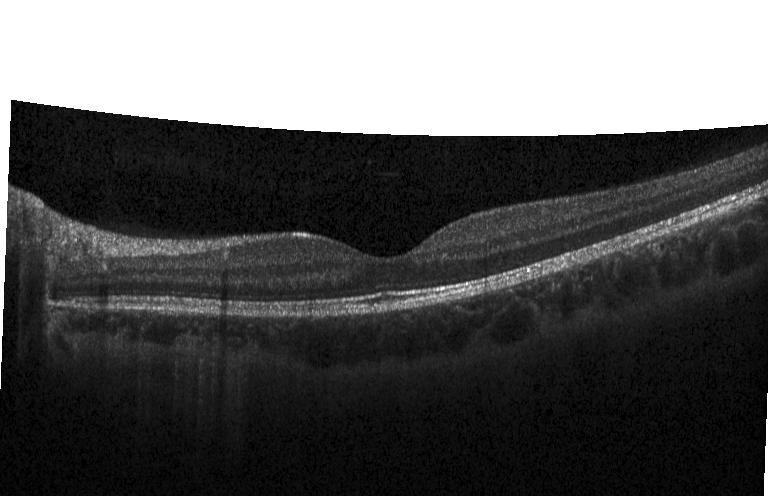
Impression: neither CNV, DME, nor drusen.